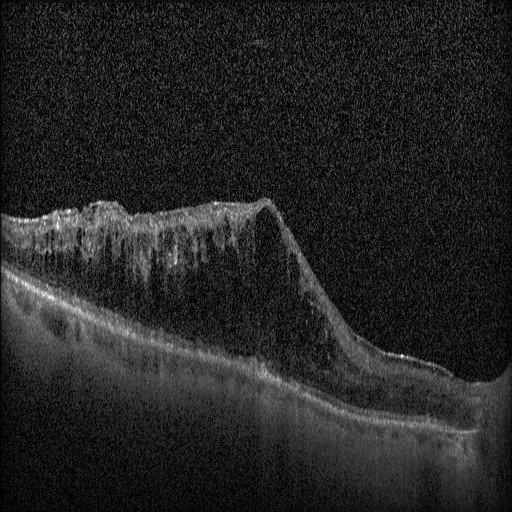

Retinal OCT cross-section showing diabetic macular edema (DME).